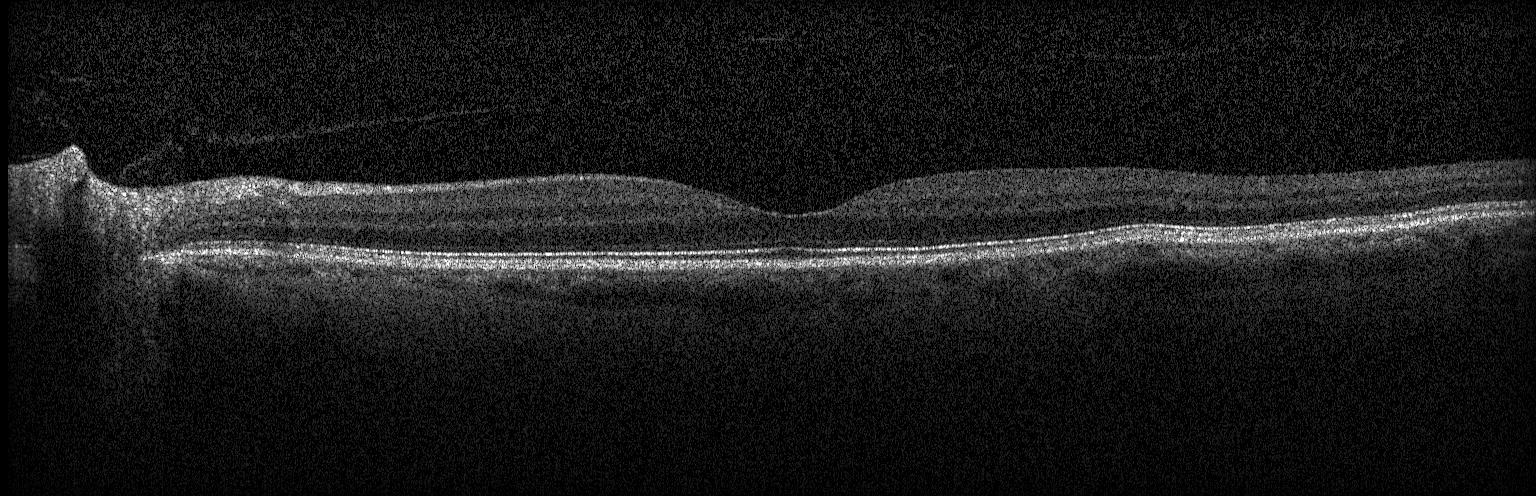

Impression: no choroidal neovascularization, no diabetic macular edema, and no drusen.